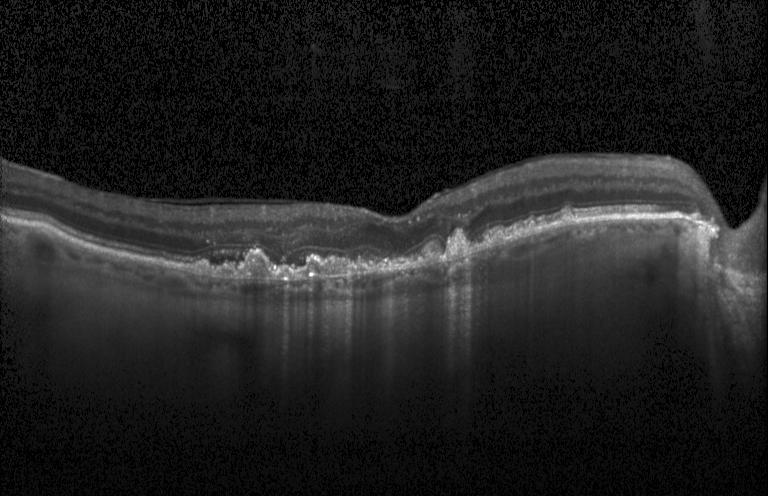

Diagnosis: choroidal neovascularization.